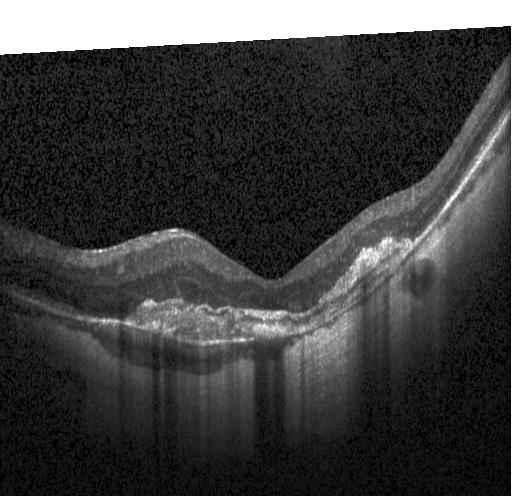 Finding: a choroidal neovascular membrane.